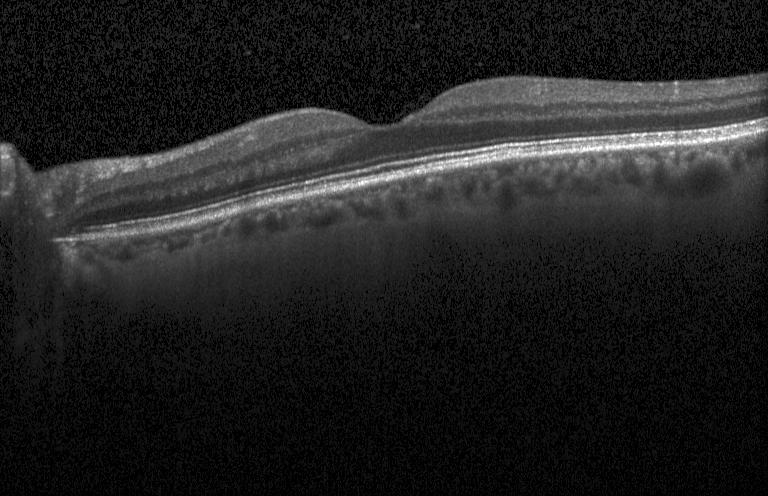 Fovea-centered. Heidelberg Spectralis. Optical coherence tomography scan. Spectral-domain optical coherence tomography — Diagnosis: no evidence of choroidal neovascularization, diabetic macular edema, or drusen.